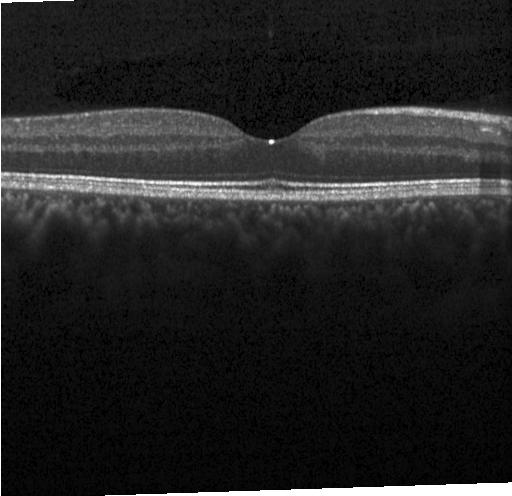 Retinal OCT cross-section — Diagnosis: no evidence of choroidal neovascularization, diabetic macular edema, or drusen.